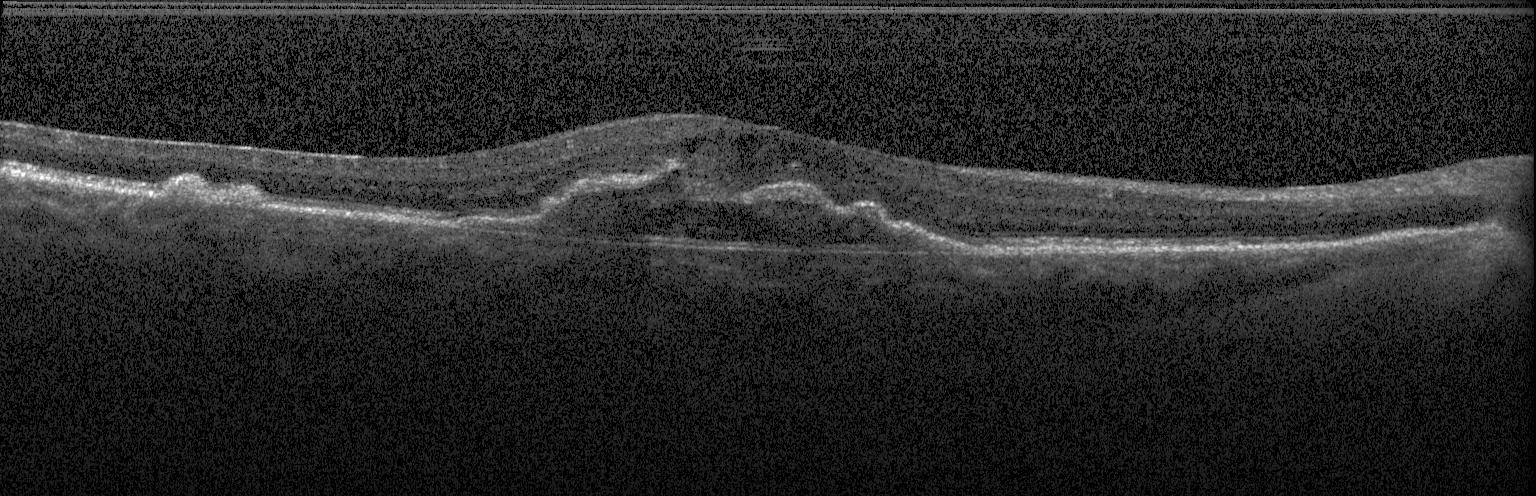

OCT line scan, acquired on a Heidelberg Spectralis, spectral-domain optical coherence tomography.
Assessment: choroidal neovascularization.